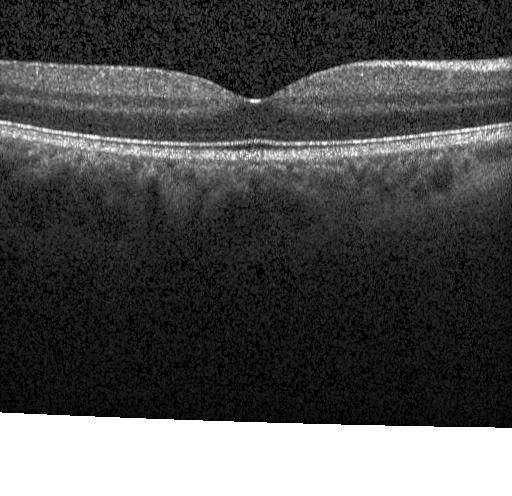

OCT line scan
Impression: no evidence of CNV, DME, or drusen.